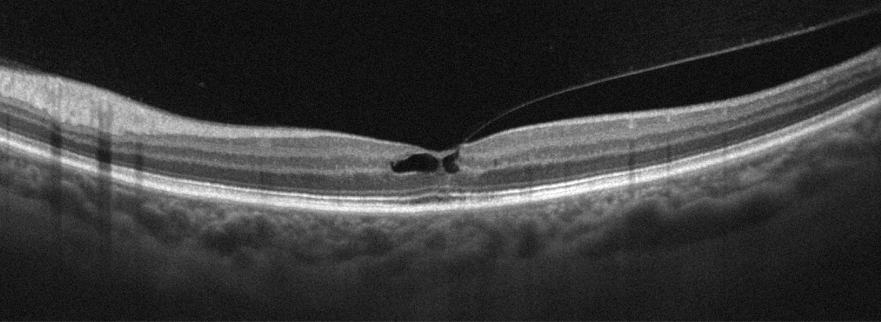

OCT finding: vitreomacular interface disease (VID).